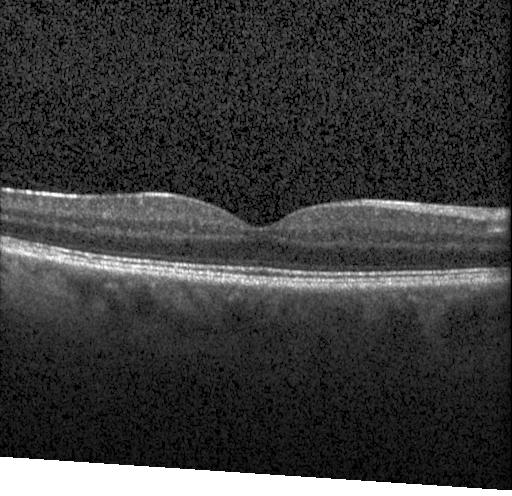
OCT B-scan. Spectral-domain OCT. Horizontal scan through the fovea — This B-scan demonstrates no evidence of CNV, DME, or drusen.